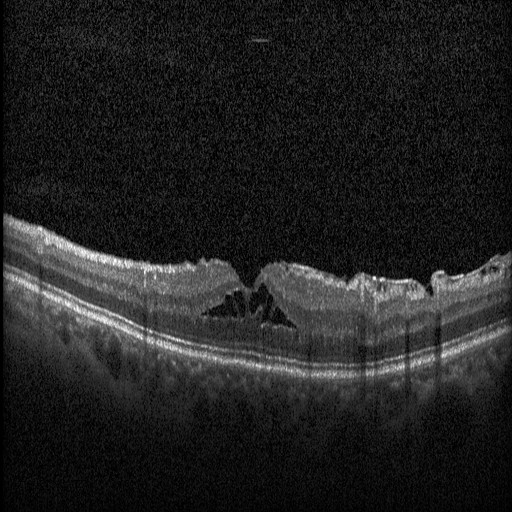
Optical coherence tomography B-scan. Fovea-centered.
The scan shows diabetic macular edema (DME).